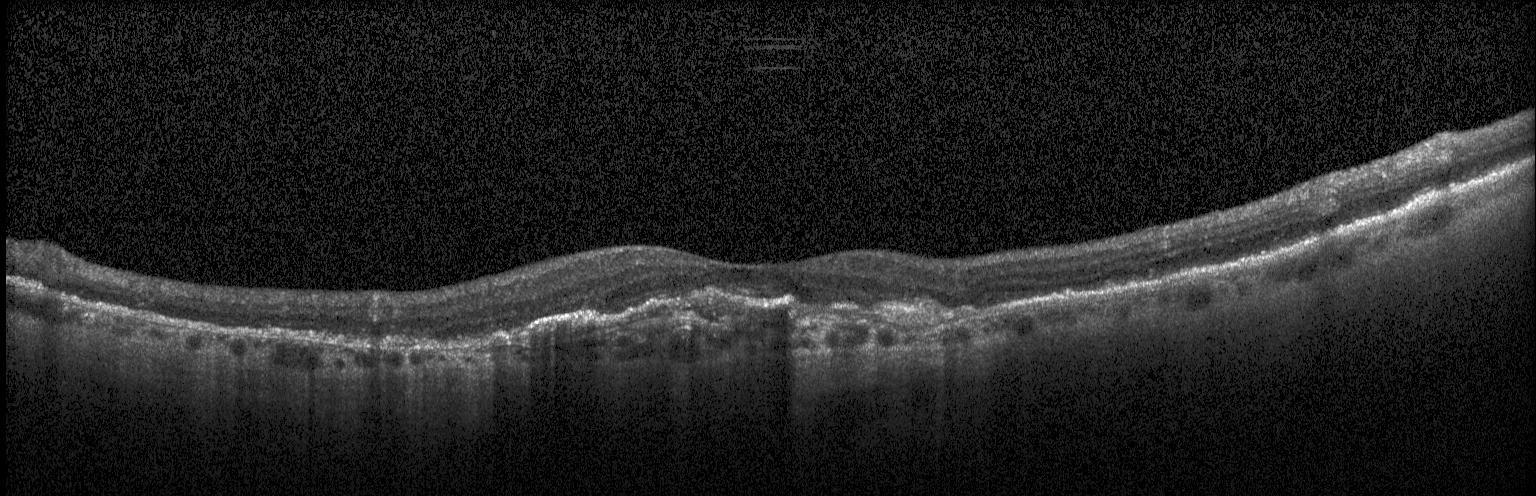 Optical coherence tomography scan. Assessment: a choroidal neovascular membrane.